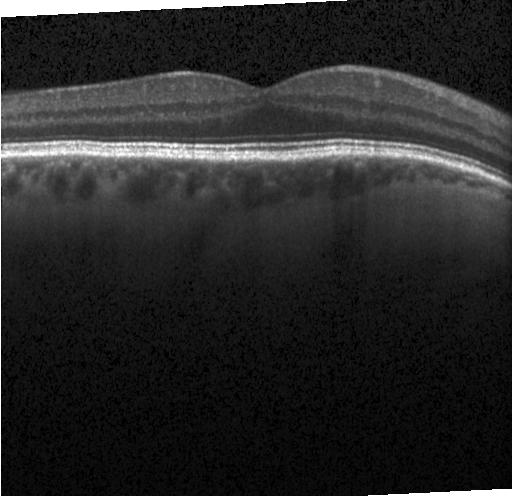
Diagnosis: no evidence of choroidal neovascularization, diabetic macular edema, or drusen.